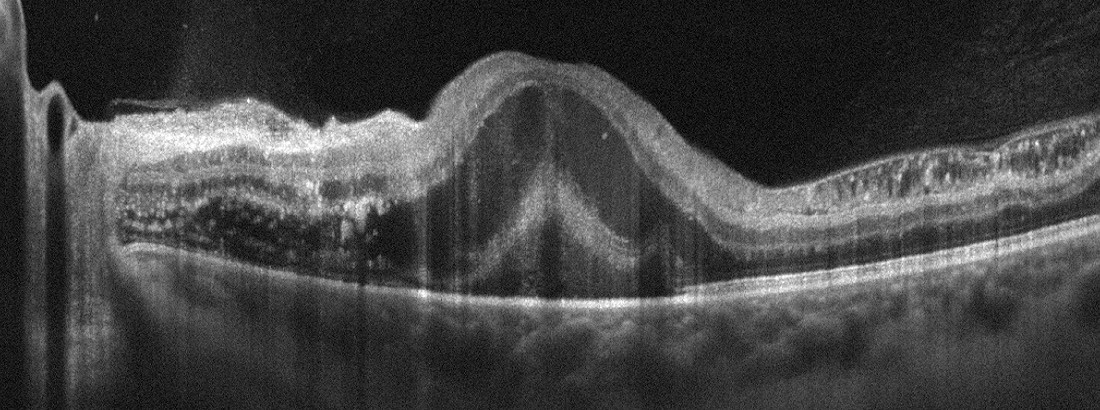
Optical coherence tomography B-scan
Diagnosis: RVO.